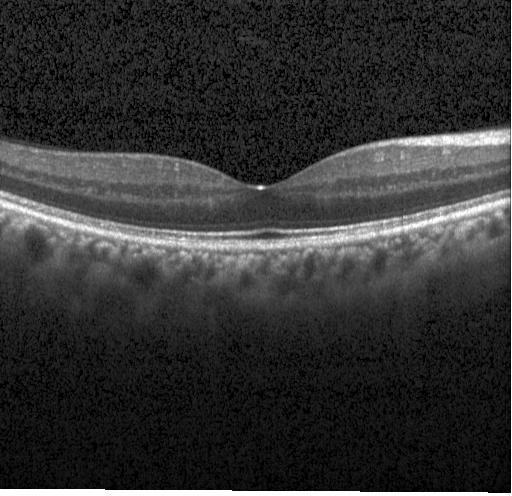

Finding: no choroidal neovascularization, diabetic macular edema, or drusen.